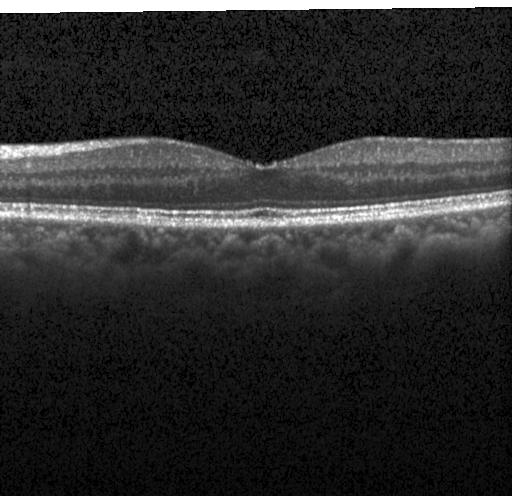

Impression: no CNV, DME, or drusen.